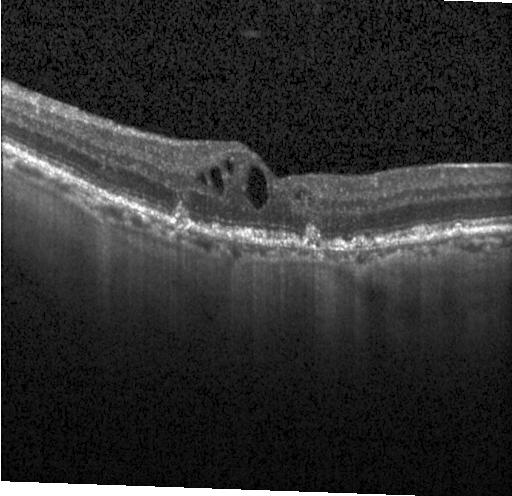

OCT finding: a choroidal neovascular membrane.